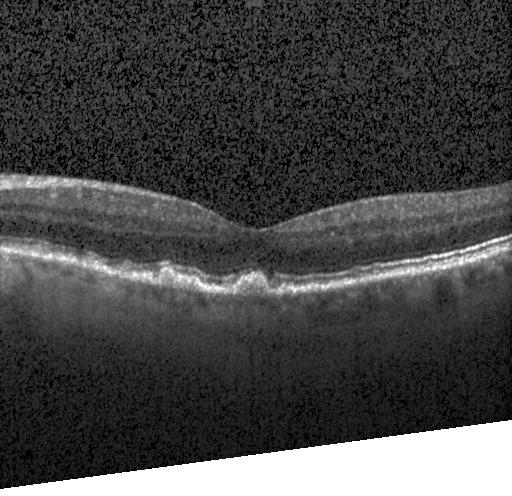
OCT line scan — OCT finding: sub-RPE drusenoid deposits.